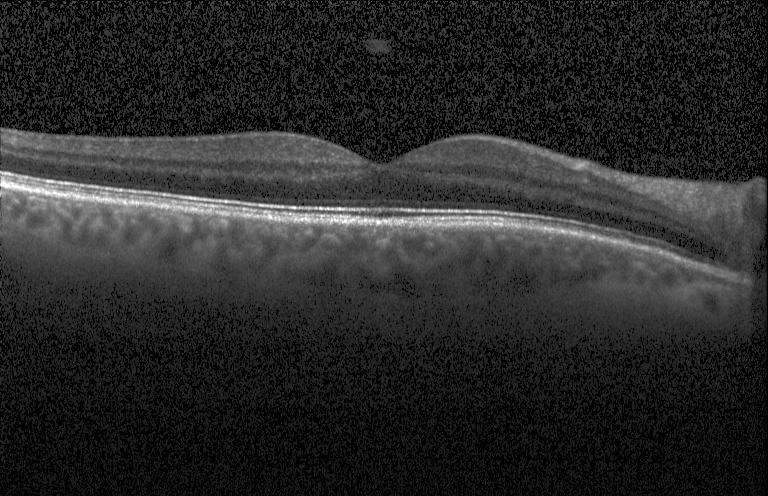
This B-scan demonstrates no evidence of choroidal neovascularization, diabetic macular edema, or drusen.